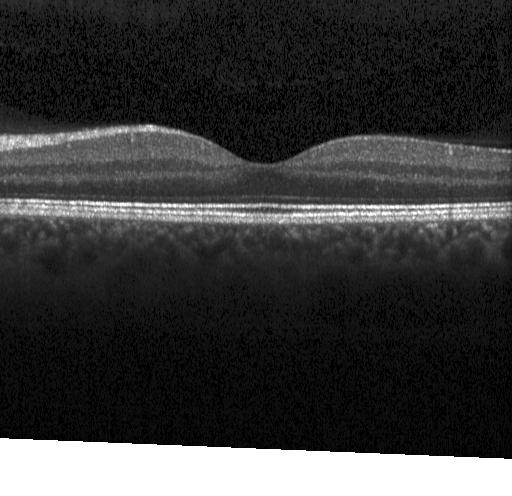 Through the macula, Heidelberg Spectralis, spectral-domain OCT, OCT B-scan.
Diagnosis: no choroidal neovascularization, diabetic macular edema, or drusen.